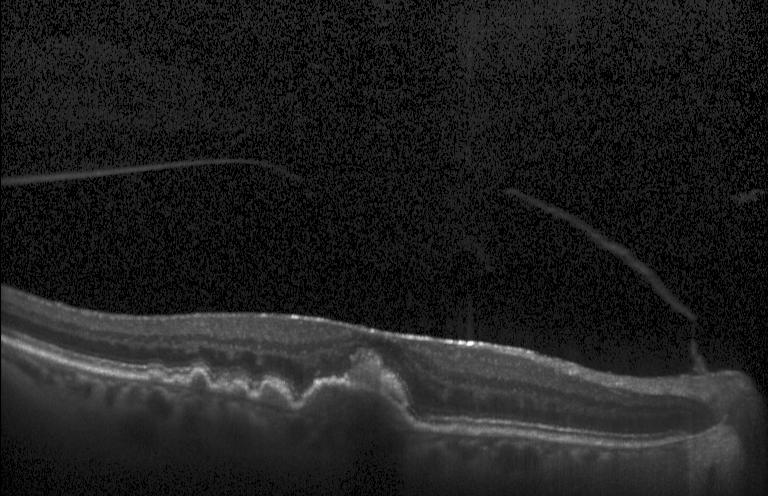 Optical coherence tomography scan · horizontal scan through the fovea — Finding: choroidal neovascularization (CNV).